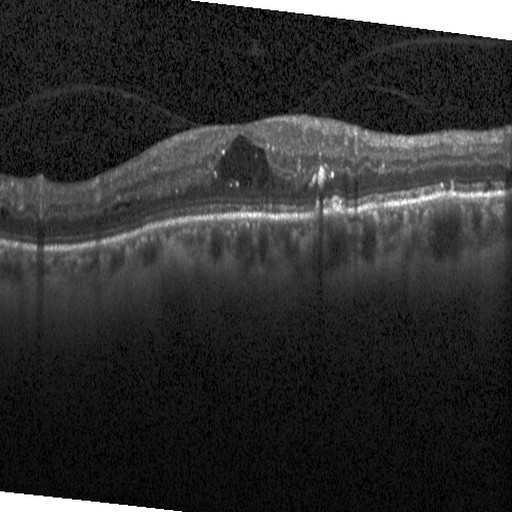 OCT line scan, instrument: Heidelberg Spectralis — The scan shows DME.